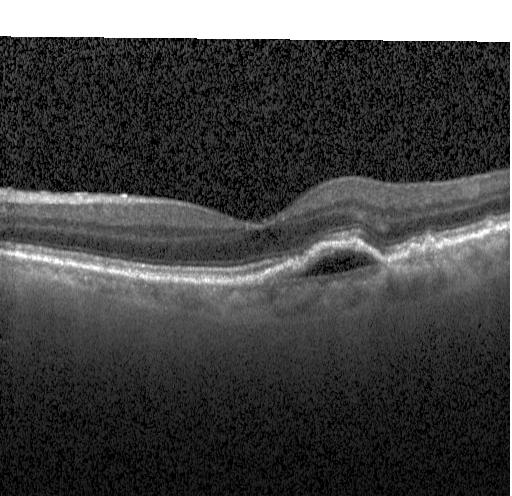 Impression: CNV.